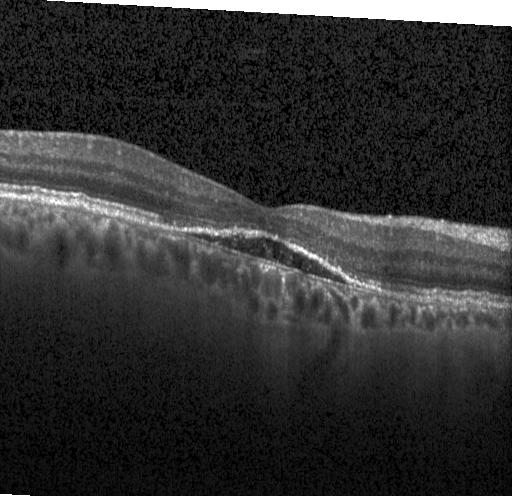

Macular OCT demonstrating a choroidal neovascular membrane.